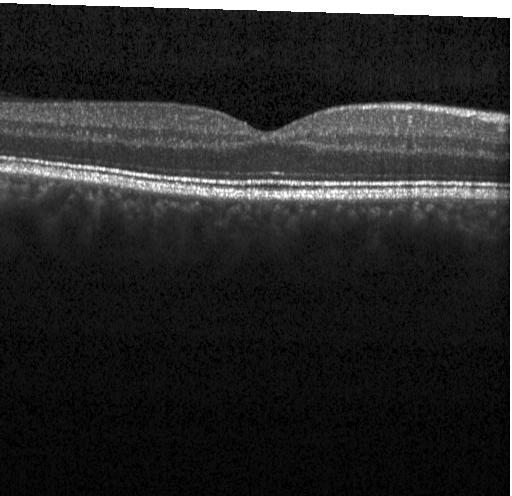
Spectral-domain OCT, OCT B-scan, instrument: Heidelberg Spectralis
This B-scan demonstrates neither choroidal neovascularization, diabetic macular edema, nor drusen.